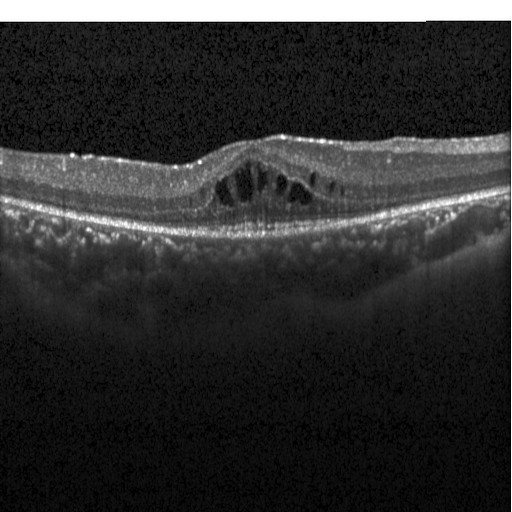 Spectral-domain OCT · through the macula · instrument: Heidelberg Spectralis · OCT line scan
Finding: DME.